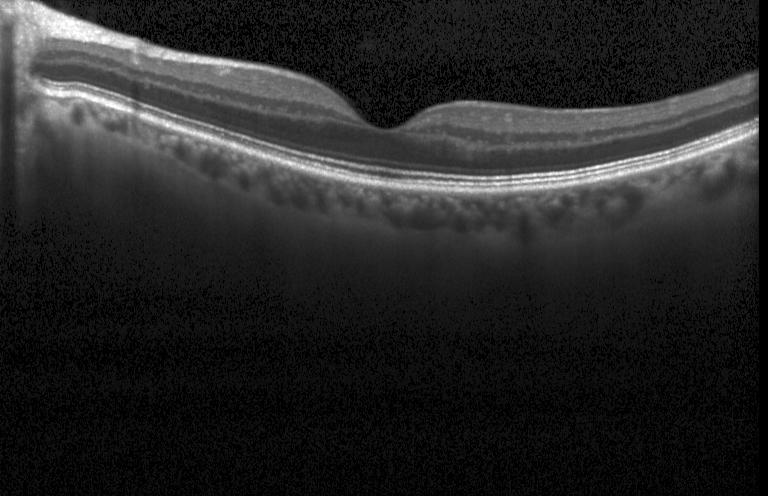

Retinal OCT B-scan · SD-OCT. This B-scan demonstrates no choroidal neovascularization, no diabetic macular edema, and no drusen.